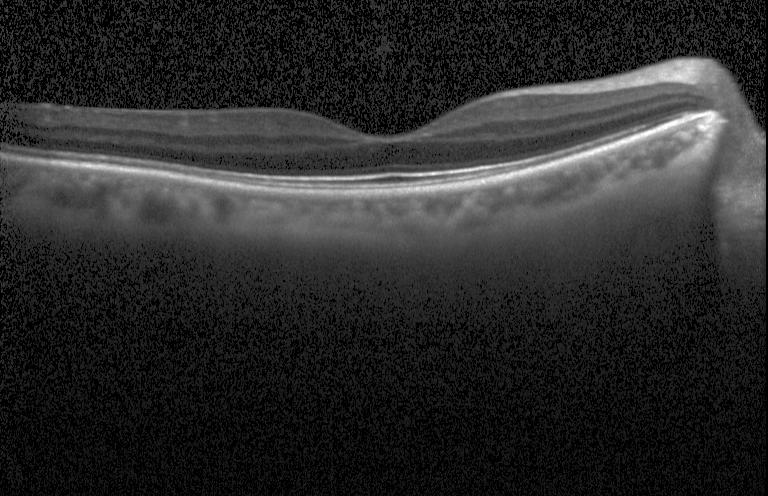 Acquired on a Heidelberg Spectralis. Optical coherence tomography scan. Fovea-centered
Diagnosis: no evidence of choroidal neovascularization, diabetic macular edema, or drusen.